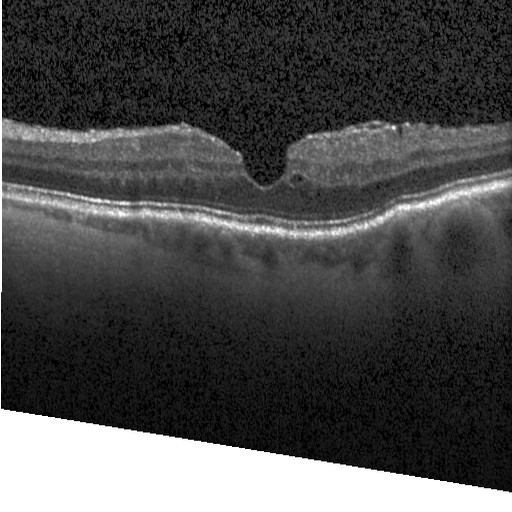 Macular scan. Retinal OCT B-scan. Instrument: Heidelberg Spectralis. OCT finding: diabetic macular edema (DME).